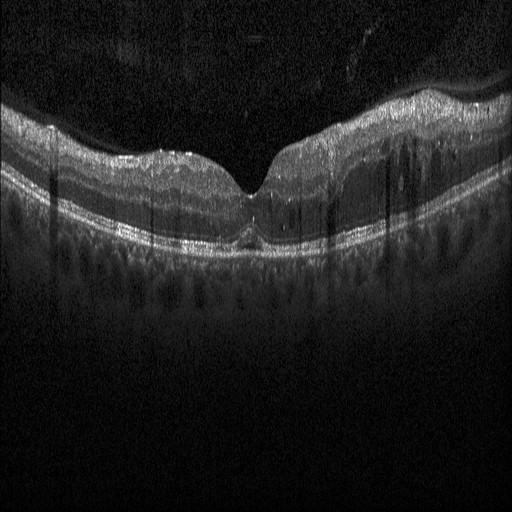
OCT line scan. Diagnosis: diabetic macular edema.